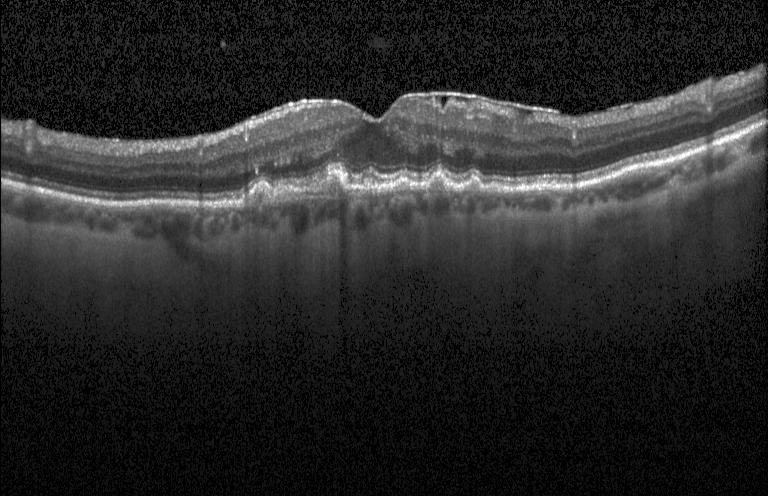
OCT scan showing drusen.